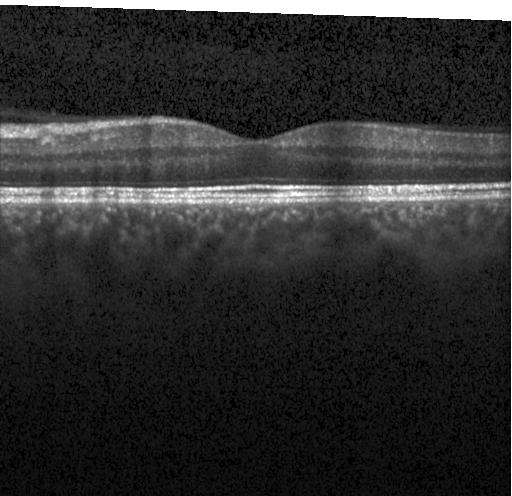
Optical coherence tomography scan.
Diagnosis: no CNV, DME, or drusen.